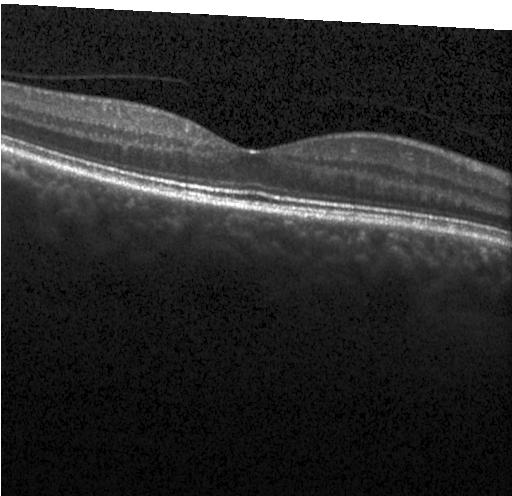

Dx: no CNV, DME, or drusen.